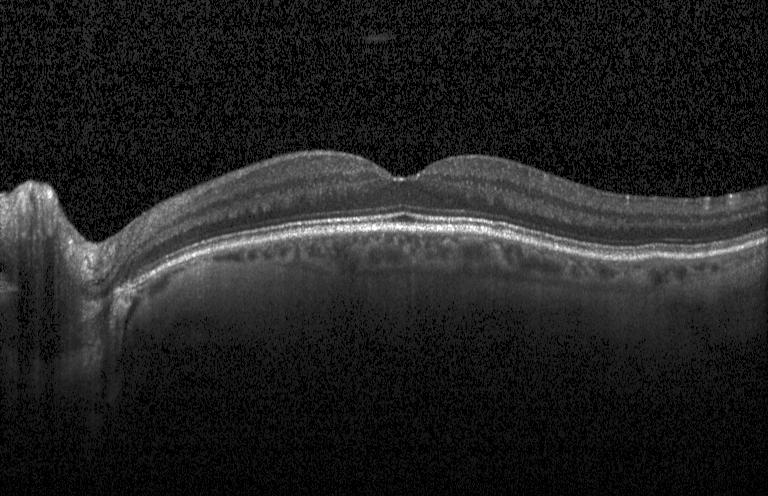 Through the macula. OCT line scan. Instrument: Heidelberg Spectralis. Spectral-domain optical coherence tomography — Finding: no evidence of CNV, DME, or drusen.